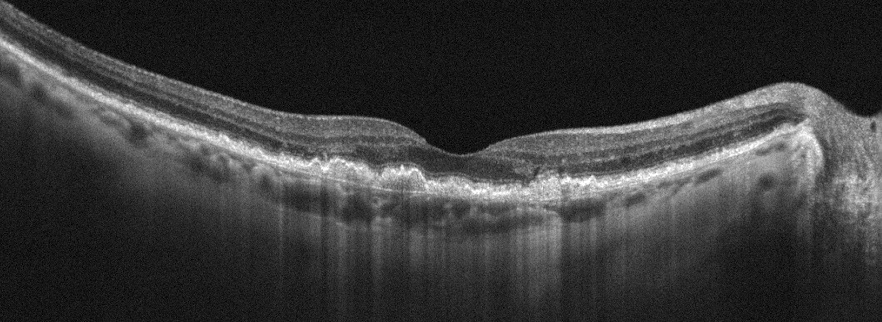

OCT scan showing age-related macular degeneration (AMD).